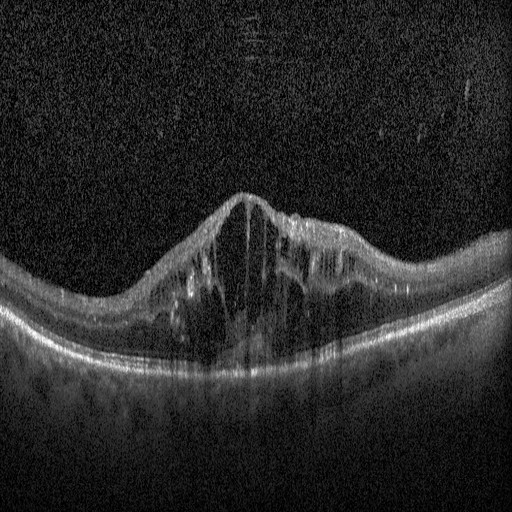

OCT B-scan showing DME.